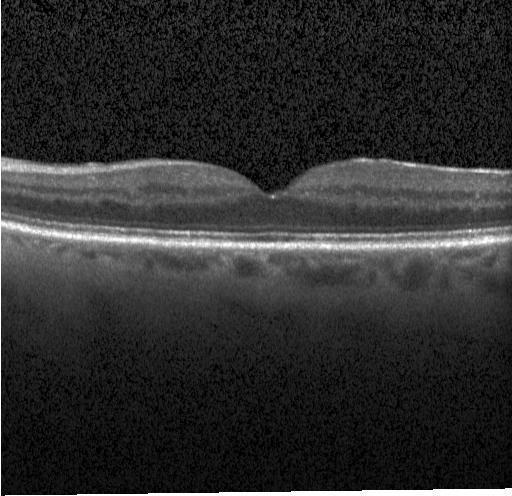 OCT finding: neither CNV, DME, nor drusen.